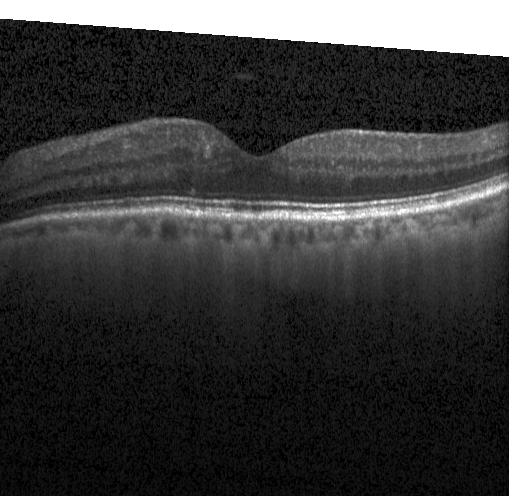
Macular scan. OCT B-scan — The scan shows no evidence of choroidal neovascularization, diabetic macular edema, or drusen.